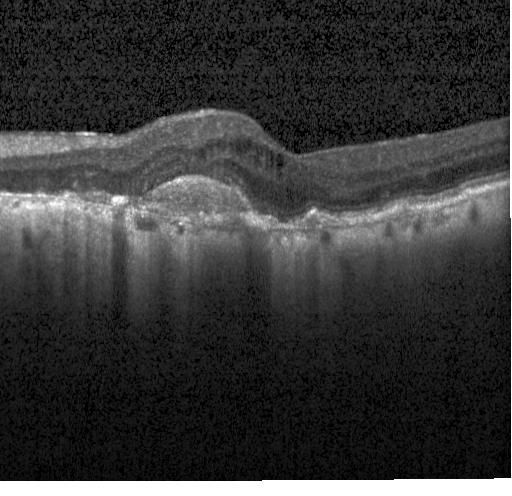 SD-OCT · Heidelberg Spectralis OCT system · retinal OCT cross-section · centered on the fovea.
OCT finding: a choroidal neovascular membrane.